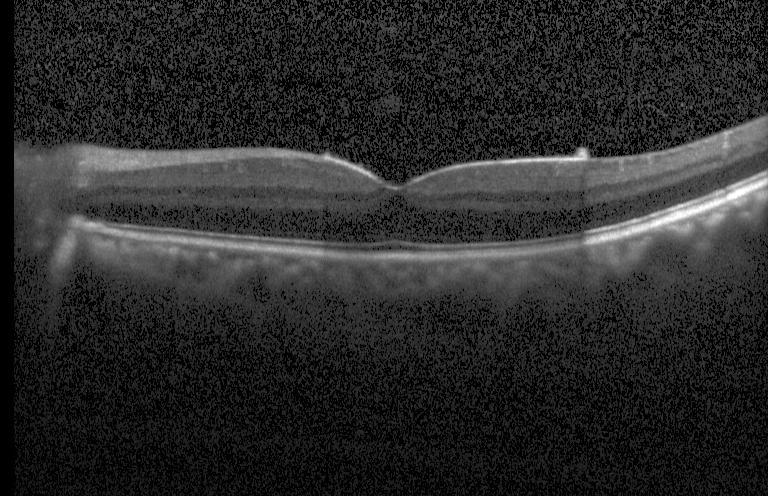

Retinal OCT B-scan — Impression: no evidence of CNV, DME, or drusen.